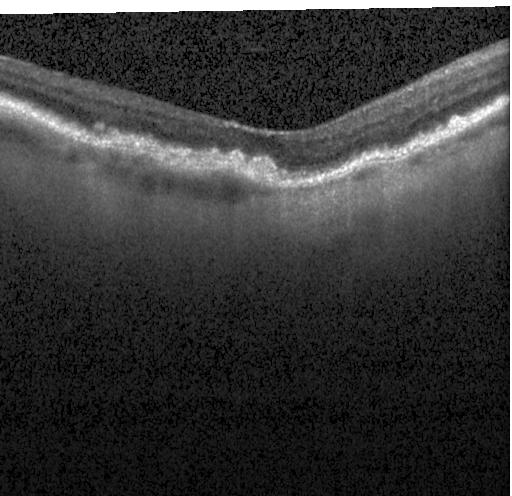
Heidelberg Spectralis OCT system. OCT line scan. Spectral-domain optical coherence tomography.
Finding: choroidal neovascularization.